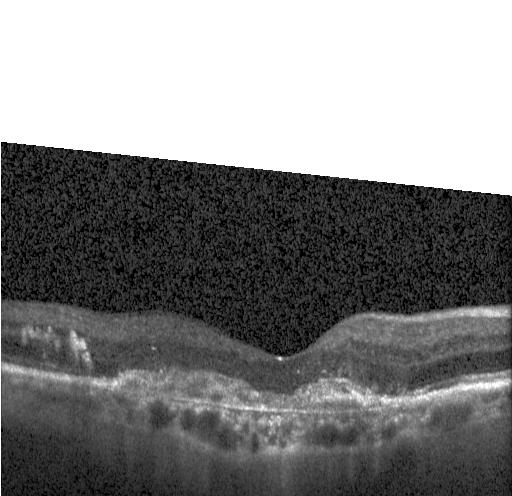 OCT B-scan showing a choroidal neovascular membrane.